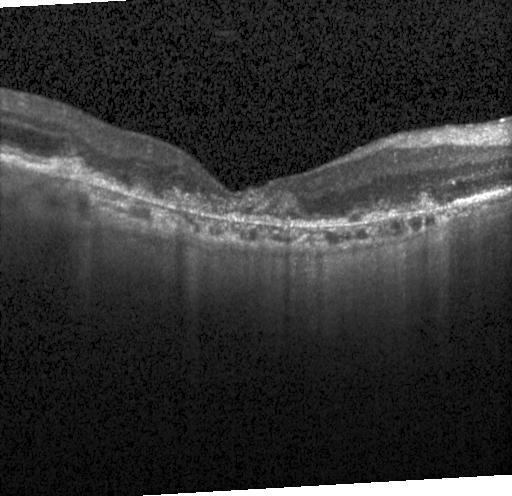

OCT finding: a choroidal neovascular membrane.